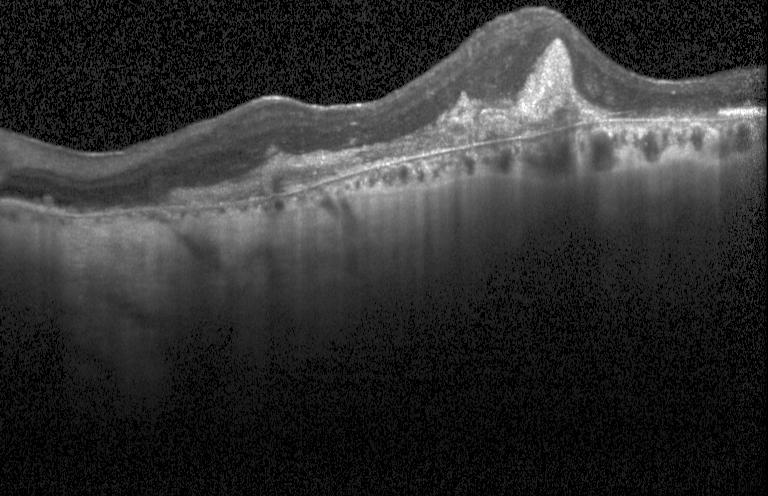
Finding: a choroidal neovascular membrane.